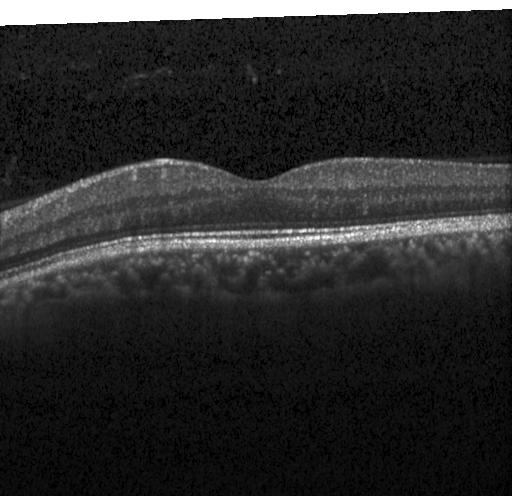 Optical coherence tomography B-scan
Macular OCT: no CNV, no DME, and no drusen.